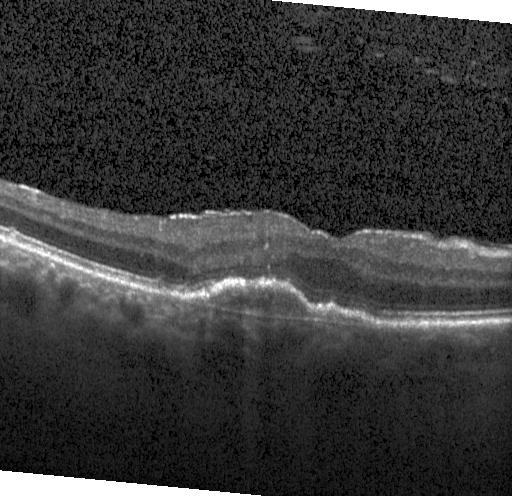

OCT B-scan showing a choroidal neovascular membrane.